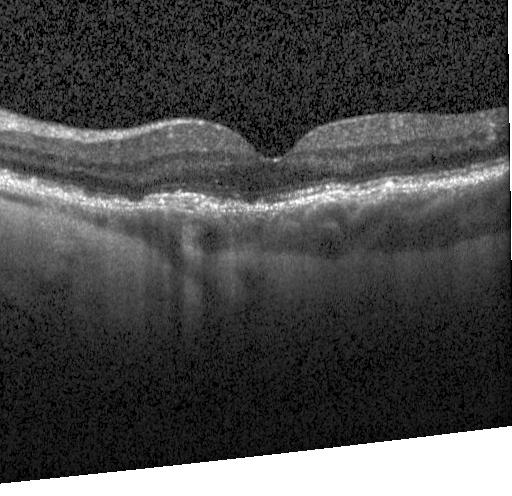 Spectral-domain optical coherence tomography, retinal OCT cross-section
Finding: a choroidal neovascular membrane.